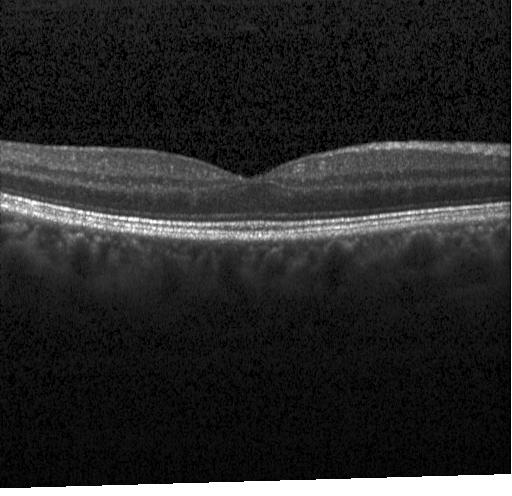 Impression: no evidence of CNV, DME, or drusen.